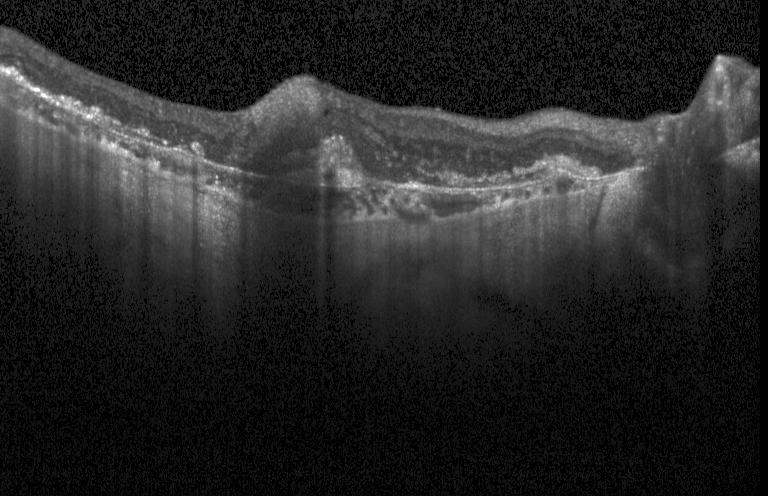 Fovea-centered · optical coherence tomography scan.
This B-scan demonstrates a choroidal neovascular membrane.